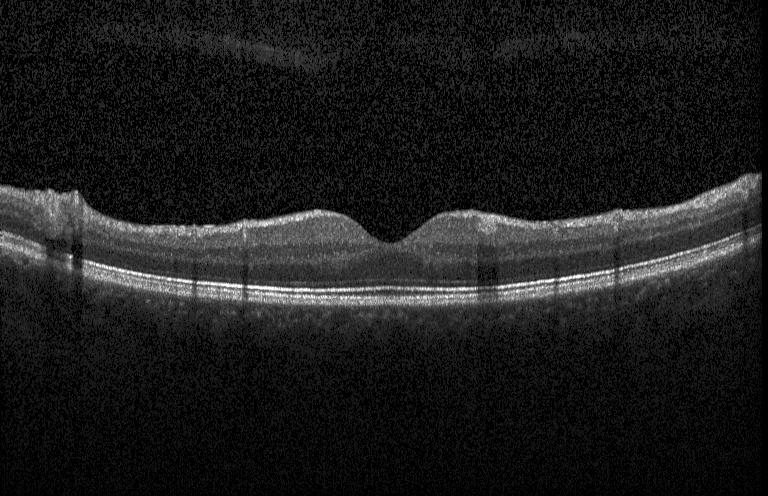

SD-OCT · macular scan · optical coherence tomography B-scan · instrument: Heidelberg Spectralis.
Dx: no choroidal neovascularization, diabetic macular edema, or drusen.